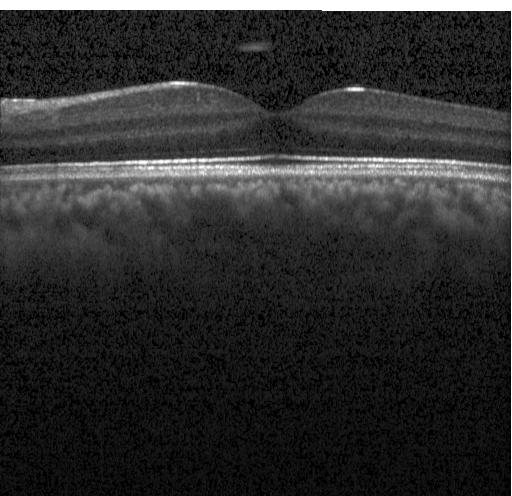
Spectral-domain optical coherence tomography. Macular scan. OCT B-scan. Heidelberg Spectralis — Diagnosis: no choroidal neovascularization, no diabetic macular edema, and no drusen.